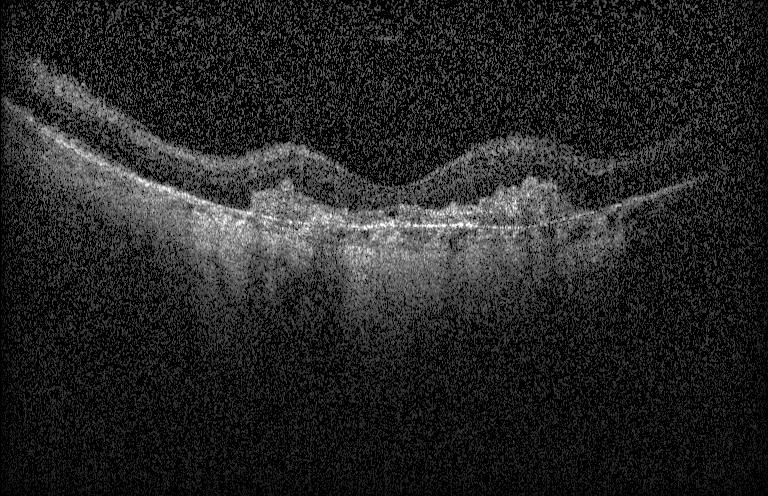 Retinal OCT cross-section — Macular OCT: a choroidal neovascular membrane.